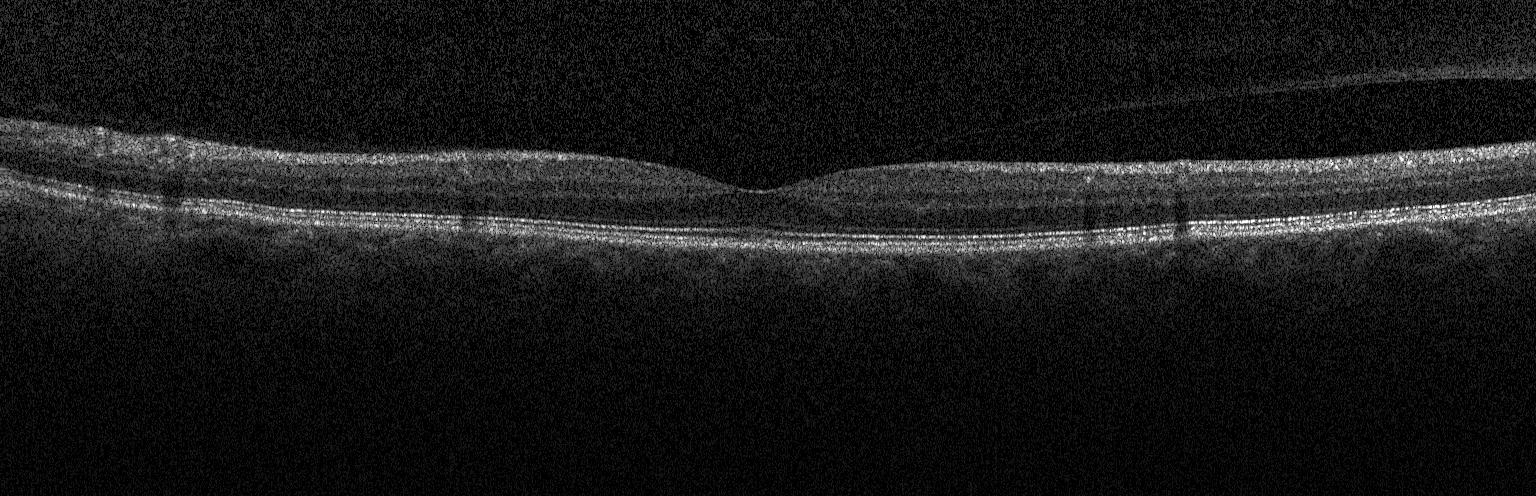

Fovea-centered. Retinal OCT B-scan — Macular OCT: neither choroidal neovascularization, diabetic macular edema, nor drusen.